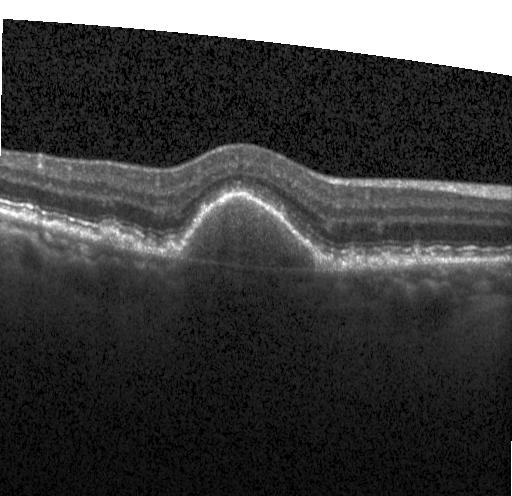
Retinal OCT B-scan; Heidelberg Spectralis — Macular OCT: a choroidal neovascular membrane.